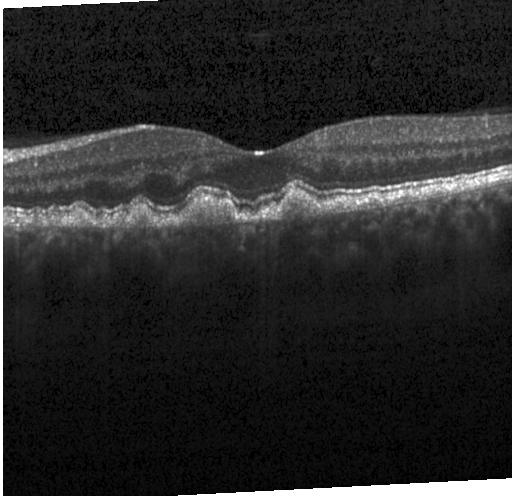
Macular OCT demonstrating sub-RPE drusenoid deposits.